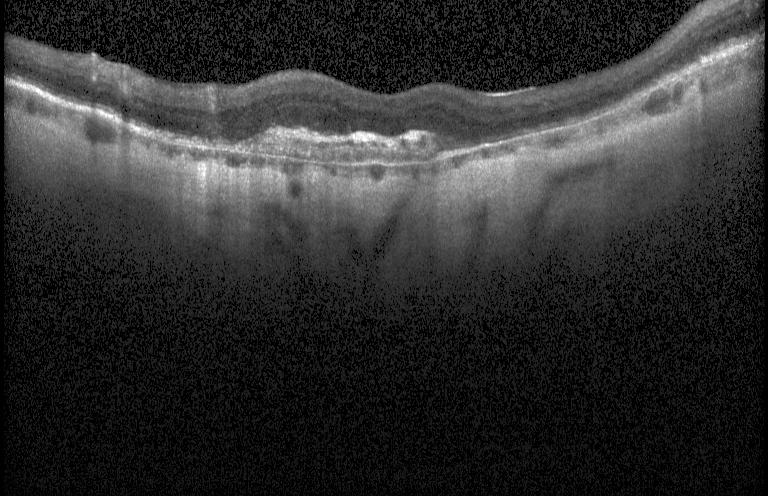

Assessment: choroidal neovascularization.